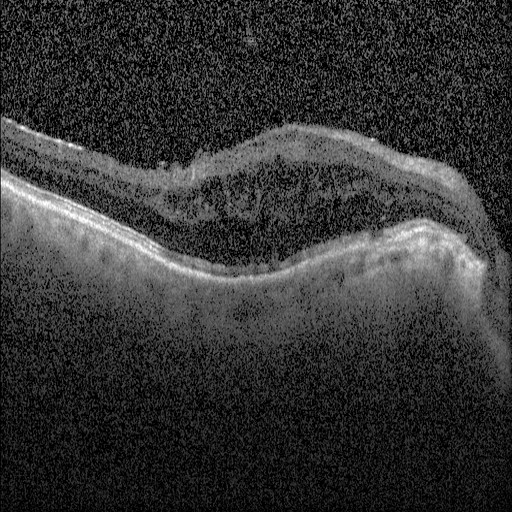
OCT finding: diabetic macular edema.